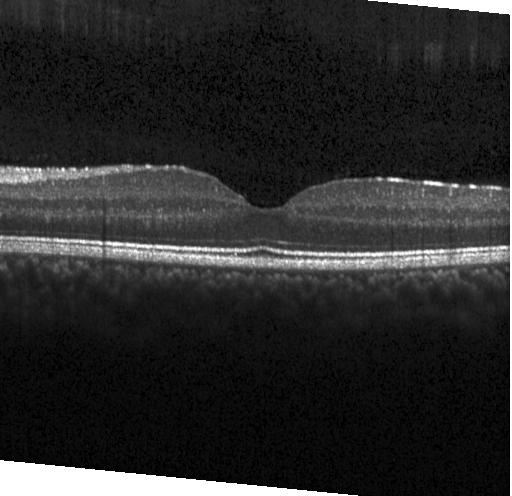
Heidelberg Spectralis. Macular scan. Spectral-domain optical coherence tomography. Retinal OCT cross-section
Neither choroidal neovascularization, diabetic macular edema, nor drusen.